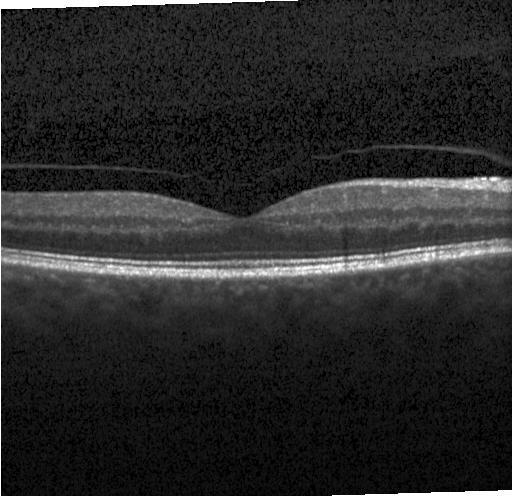

The scan shows no evidence of choroidal neovascularization, diabetic macular edema, or drusen.